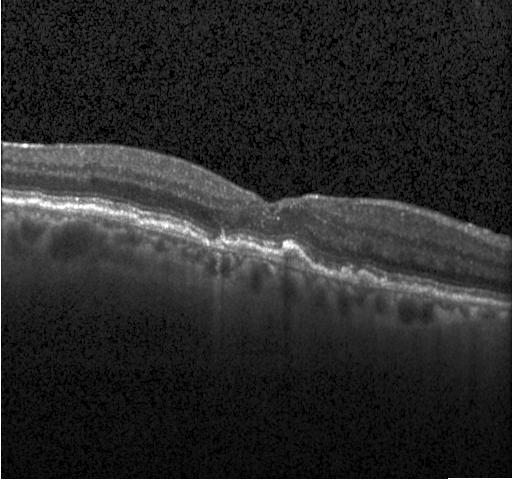
Heidelberg Spectralis · through the macula · SD-OCT · optical coherence tomography B-scan — Diagnosis: a choroidal neovascular membrane.